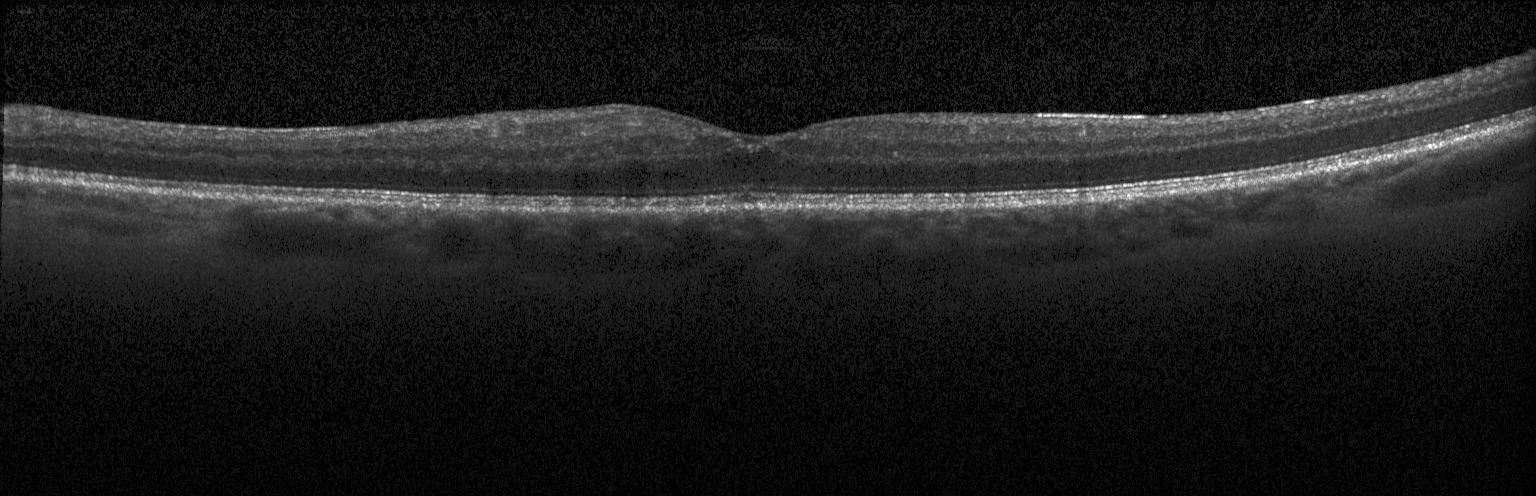

No choroidal neovascularization, no diabetic macular edema, and no drusen.